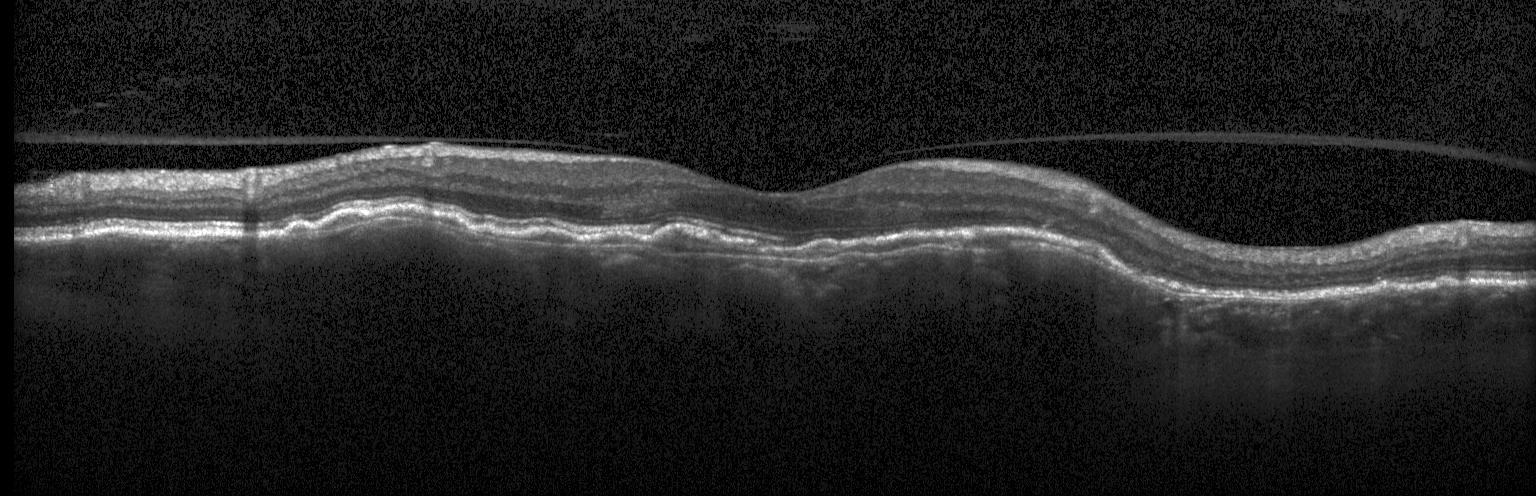

Through the macula. Retinal OCT B-scan. Instrument: Heidelberg Spectralis. Assessment: a choroidal neovascular membrane.